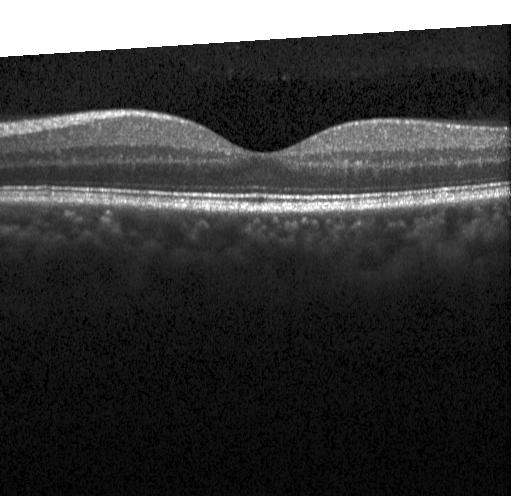

OCT line scan. Heidelberg Spectralis. OCT finding: no evidence of choroidal neovascularization, diabetic macular edema, or drusen.